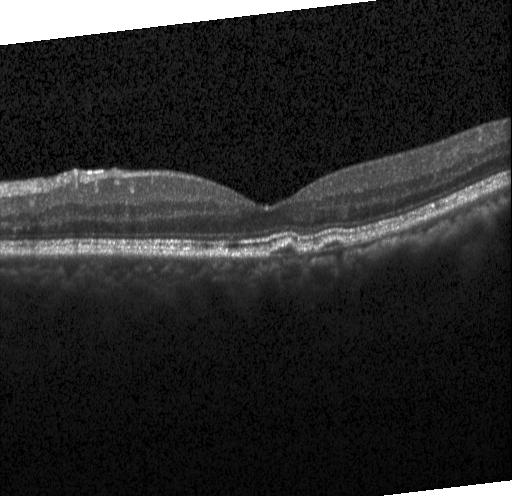

Retinal OCT cross-section showing sub-RPE drusenoid deposits.